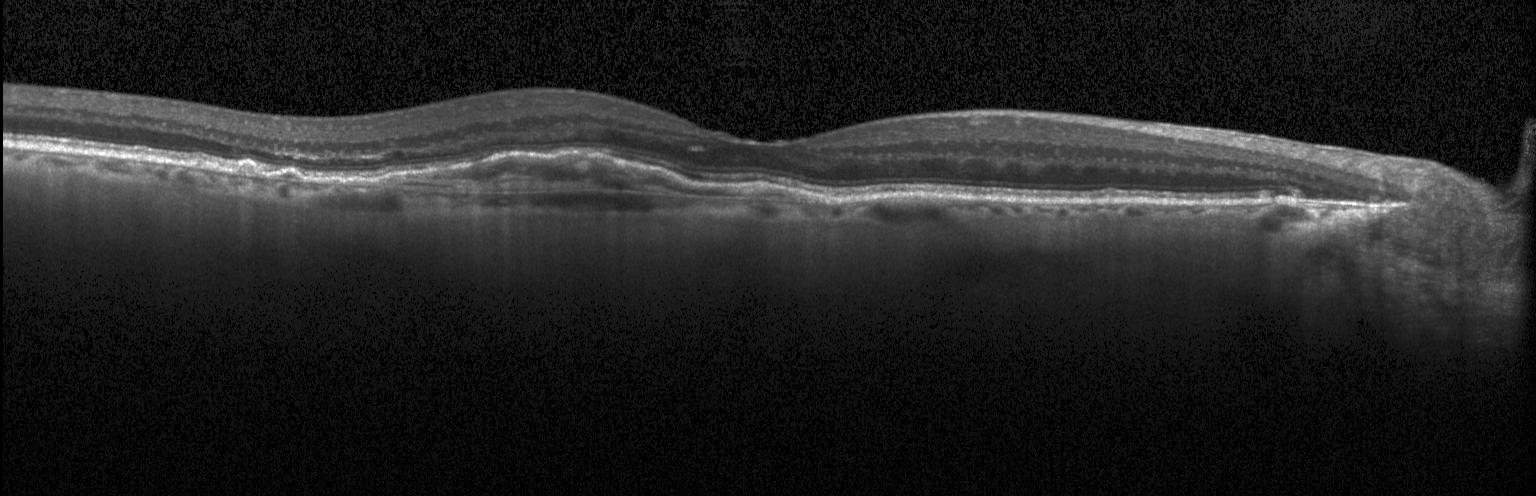

Heidelberg Spectralis · OCT line scan · spectral-domain OCT · macular scan.
Dx: a choroidal neovascular membrane.